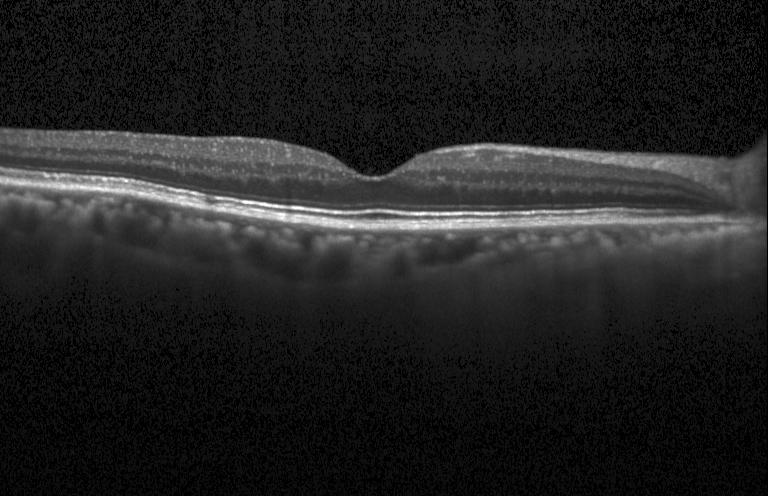 Optical coherence tomography B-scan.
Diagnosis: no evidence of choroidal neovascularization, diabetic macular edema, or drusen.